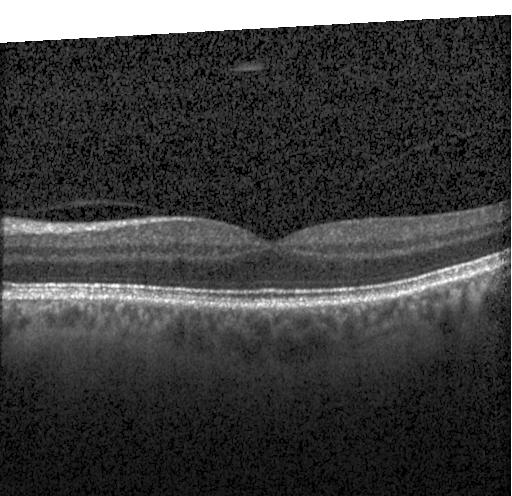

OCT B-scan showing no evidence of CNV, DME, or drusen.